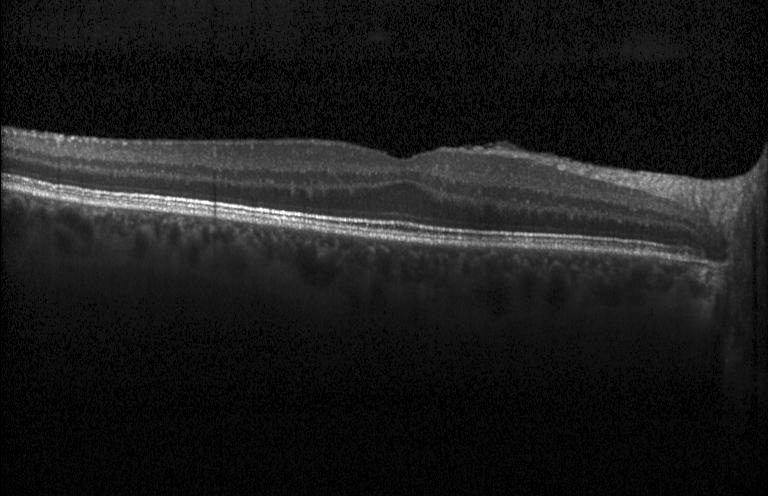
OCT line scan — Finding: no choroidal neovascularization, diabetic macular edema, or drusen.